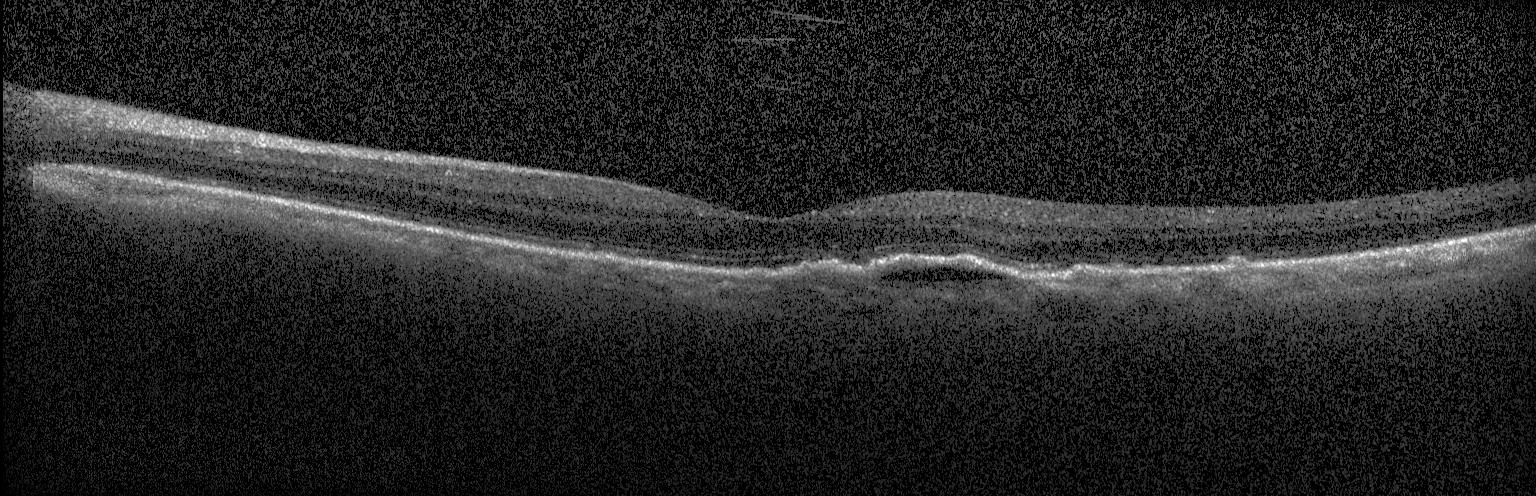
Through the macula. Optical coherence tomography scan. Spectral-domain optical coherence tomography. Heidelberg Spectralis OCT system.
Impression: choroidal neovascularization.